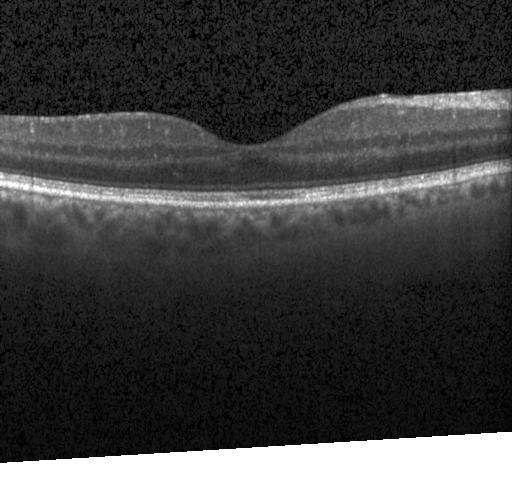
Heidelberg Spectralis OCT system; optical coherence tomography B-scan; horizontal scan through the fovea.
Diagnosis: no CNV, no DME, and no drusen.